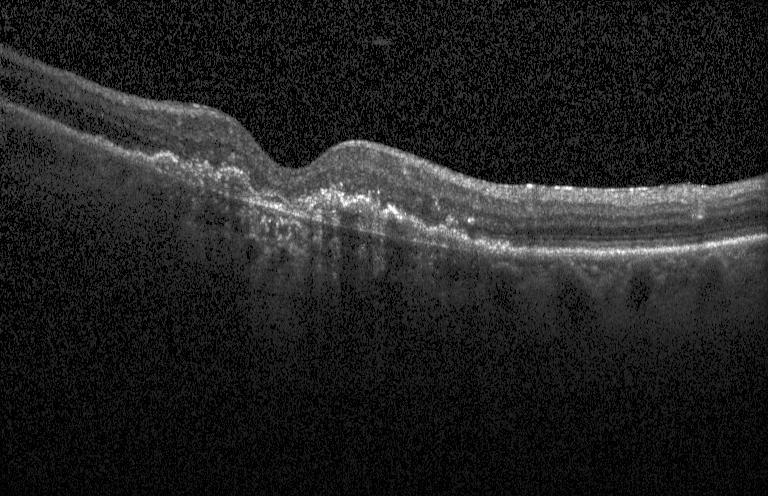 Retinal OCT B-scan — Diagnosis: a choroidal neovascular membrane.